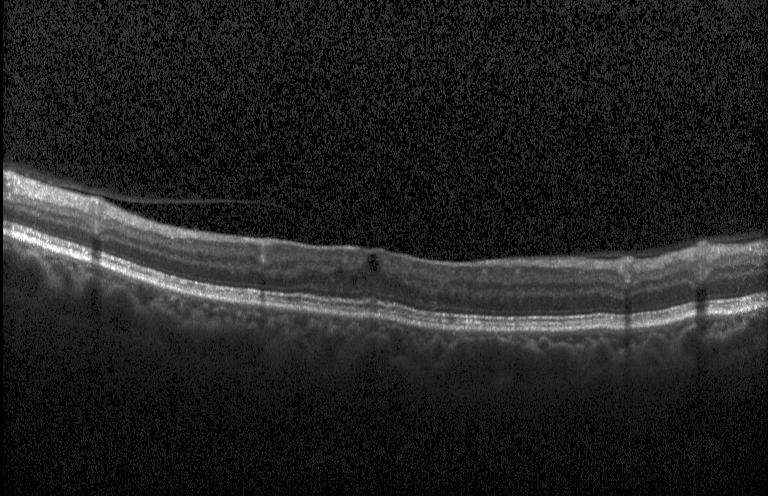
Retinal OCT B-scan; Heidelberg Spectralis; fovea-centered; SD-OCT.
Finding: diabetic macular edema (DME).